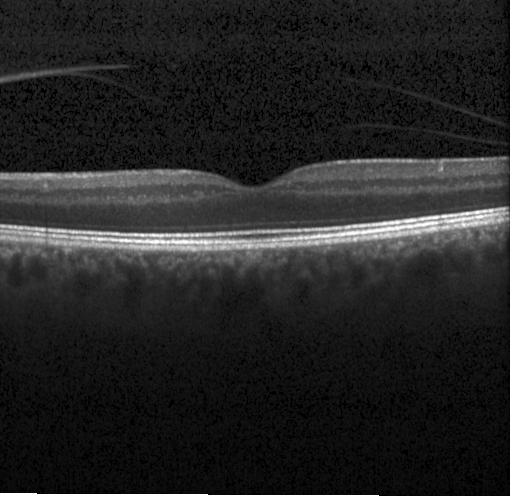
Macular OCT demonstrating no evidence of choroidal neovascularization, diabetic macular edema, or drusen.